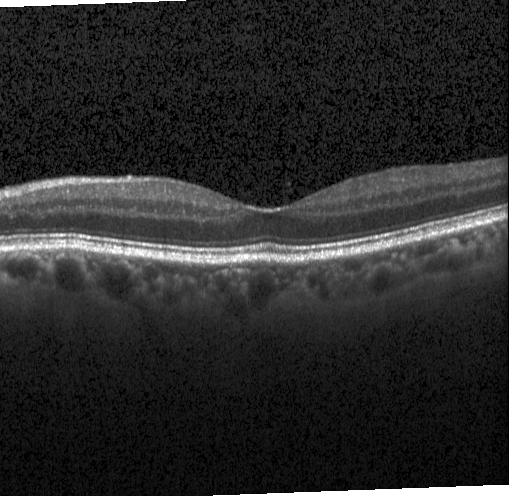
SD-OCT, instrument: Heidelberg Spectralis, optical coherence tomography B-scan
The scan shows no CNV, no DME, and no drusen.